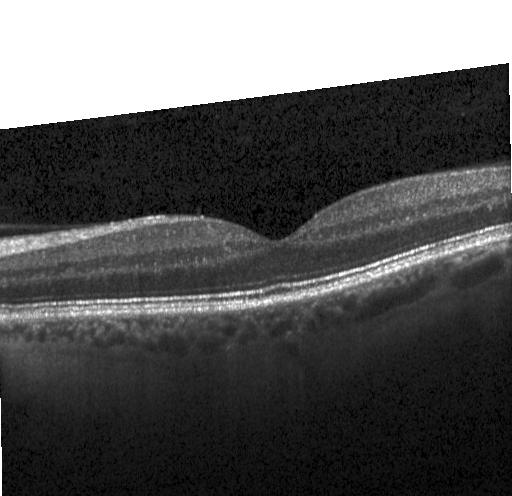 Macular OCT demonstrating neither CNV, DME, nor drusen.